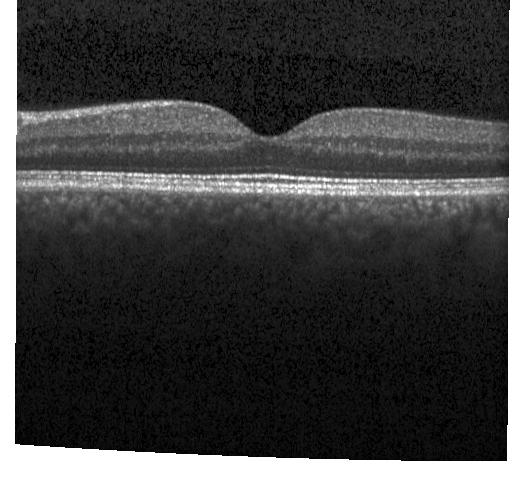

Centered on the fovea · acquired on a Heidelberg Spectralis · retinal OCT B-scan. Diagnosis: no choroidal neovascularization, no diabetic macular edema, and no drusen.